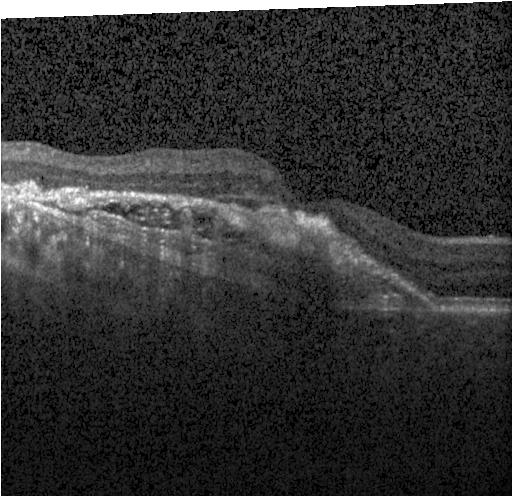 Acquired on a Heidelberg Spectralis, optical coherence tomography B-scan, through the macula. OCT finding: a choroidal neovascular membrane.